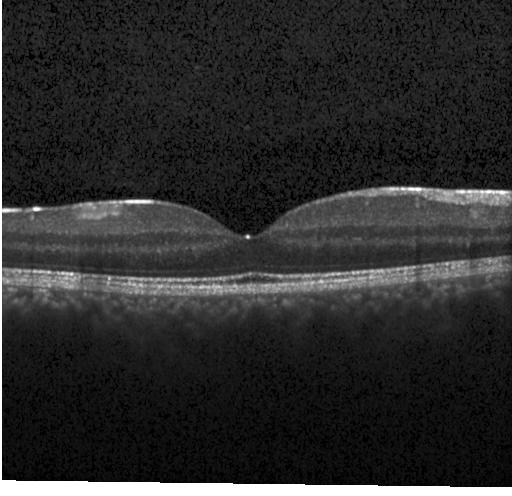 OCT B-scan. This B-scan demonstrates no choroidal neovascularization, diabetic macular edema, or drusen.